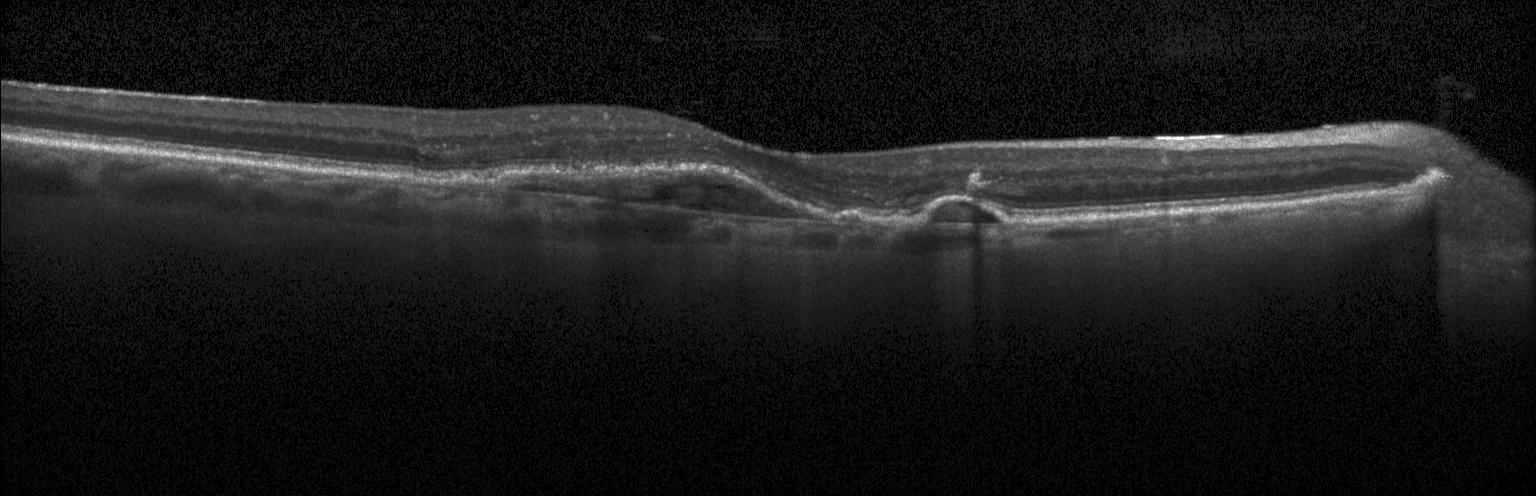
Finding: choroidal neovascularization (CNV).